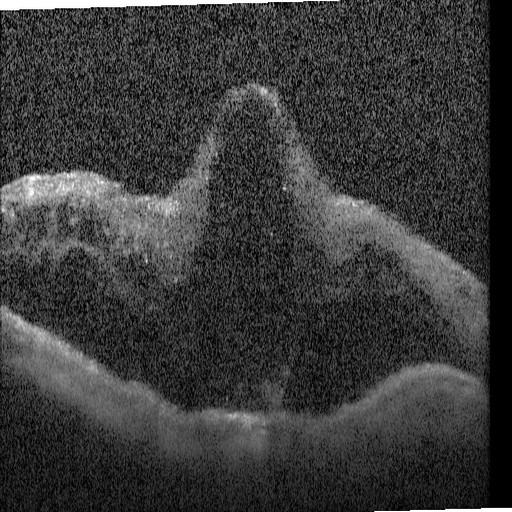
SD-OCT; OCT B-scan
Diagnosis: diabetic macular edema.